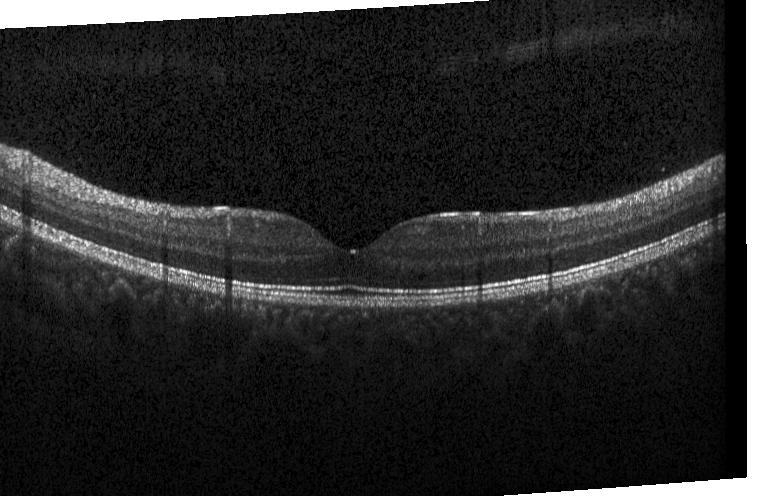
Optical coherence tomography scan.
Macular OCT: neither choroidal neovascularization, diabetic macular edema, nor drusen.